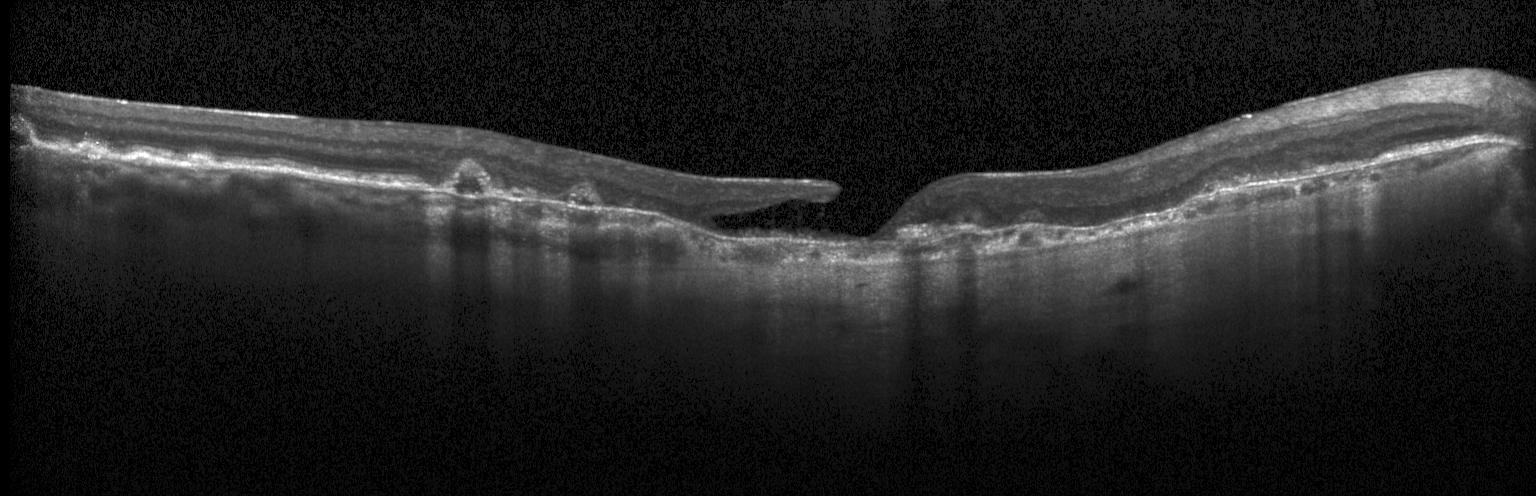 Macular scan. SD-OCT. Optical coherence tomography scan. Heidelberg Spectralis
Dx: a choroidal neovascular membrane.